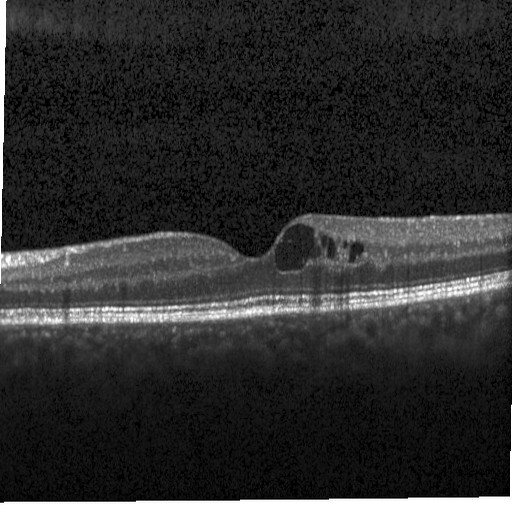

Acquired on a Heidelberg Spectralis; OCT B-scan — This B-scan demonstrates diabetic macular edema.